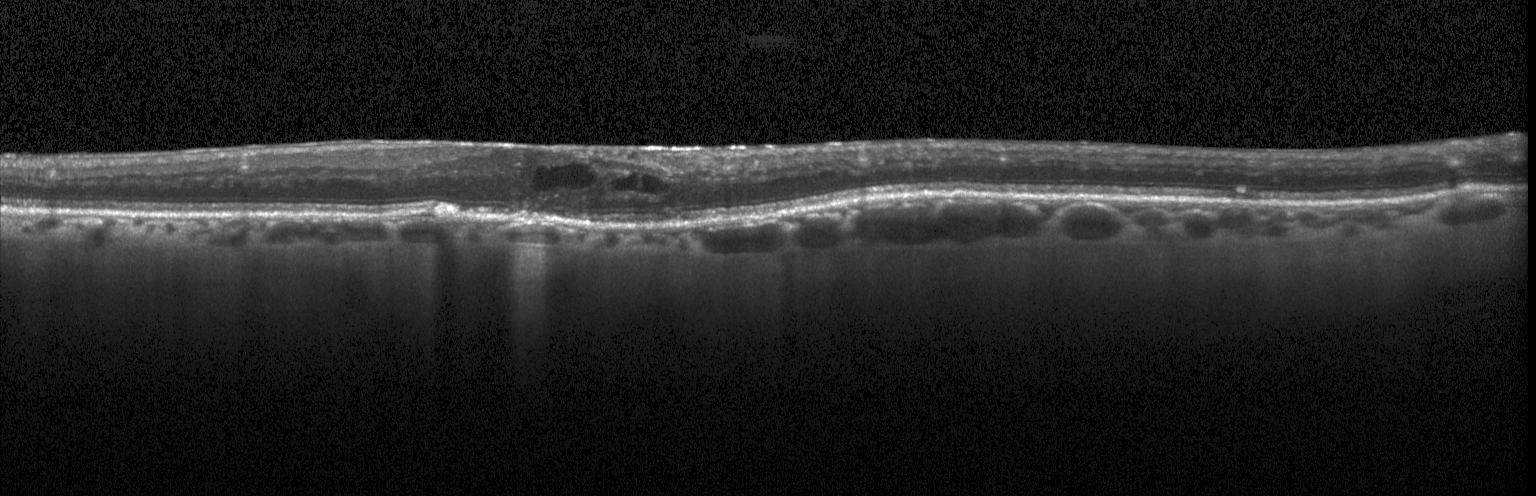
Retinal OCT cross-section showing CNV.